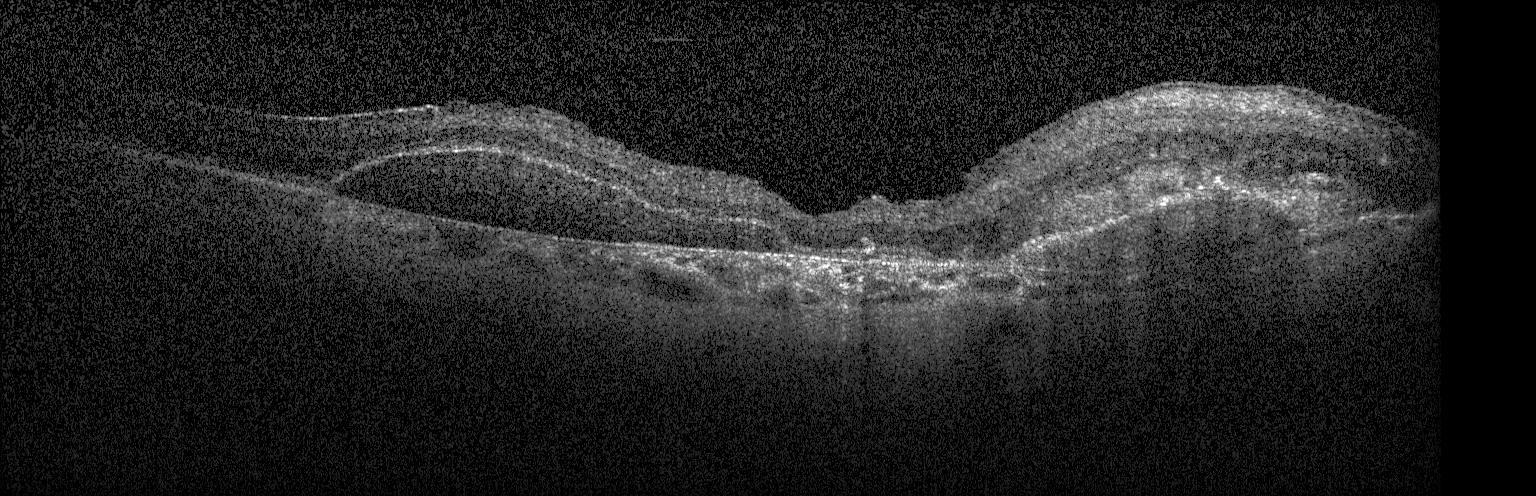

OCT B-scan · macular scan. Choroidal neovascularization.